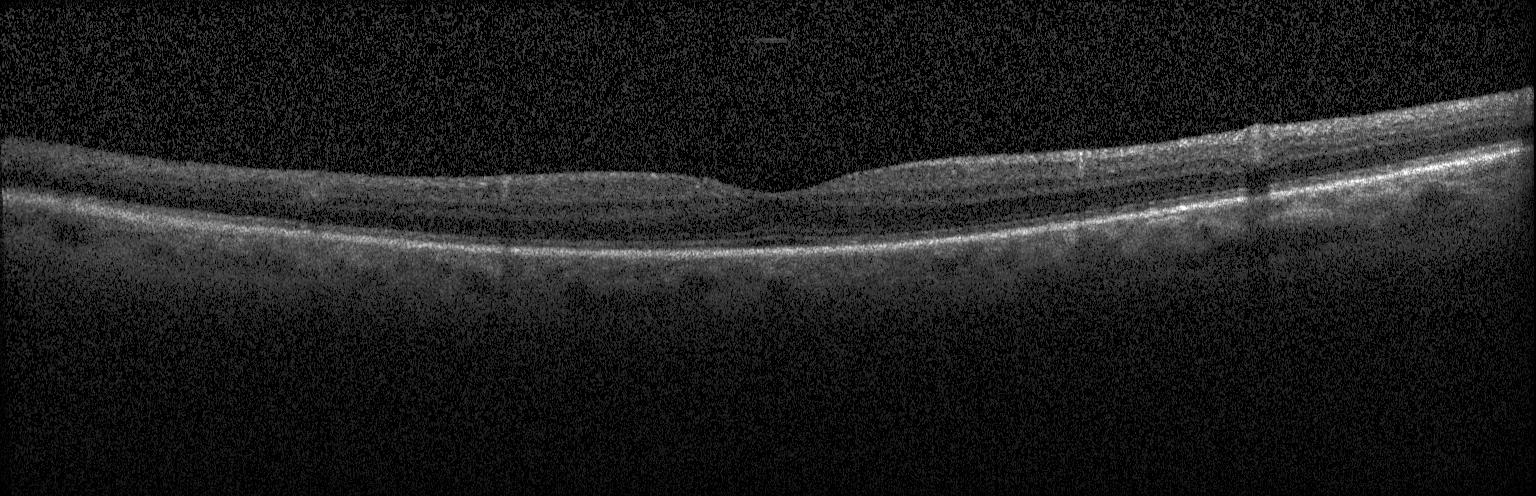

This B-scan demonstrates no CNV, no DME, and no drusen.